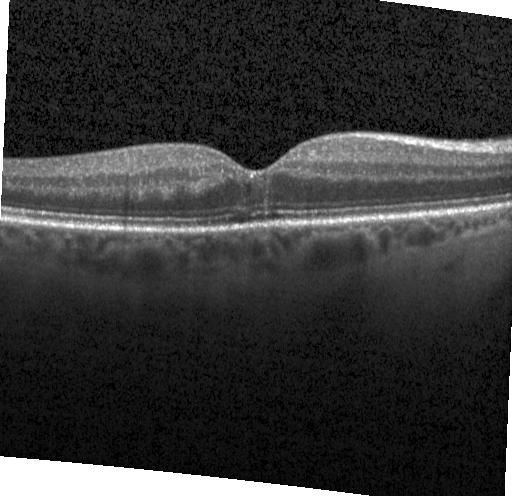
OCT B-scan; Heidelberg Spectralis; spectral-domain OCT; macular scan — Diagnosis: no CNV, DME, or drusen.